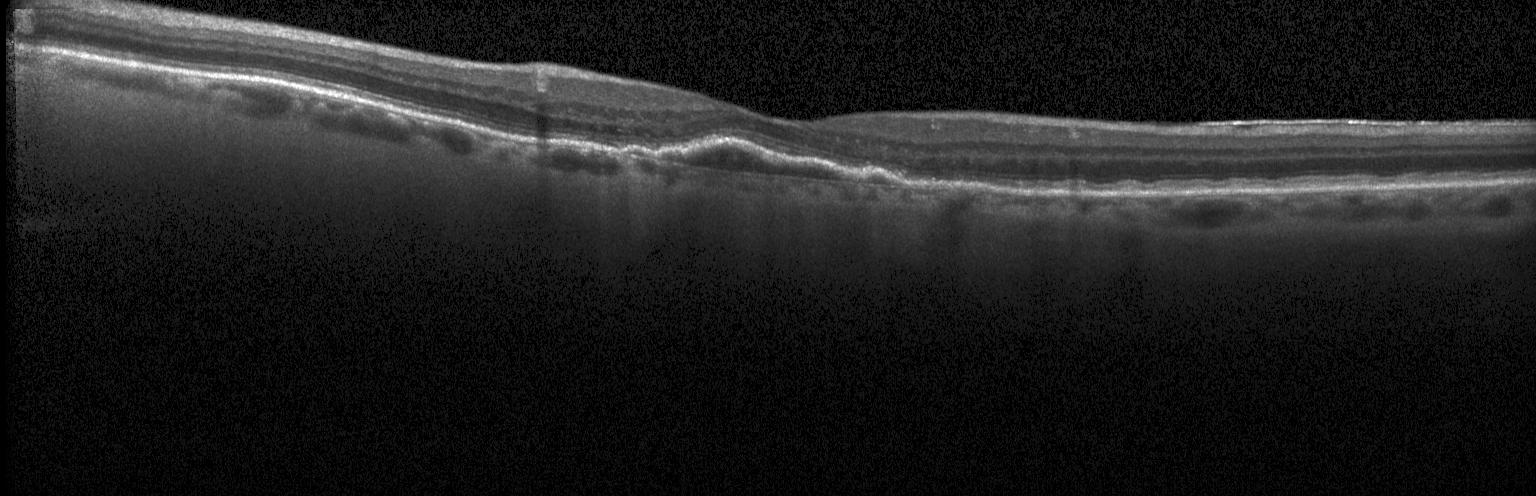
OCT scan showing choroidal neovascularization (CNV).